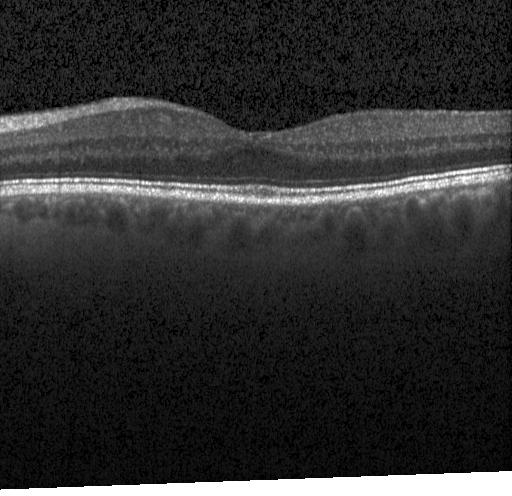

OCT line scan. Horizontal scan through the fovea. Heidelberg Spectralis. Dx: neither choroidal neovascularization, diabetic macular edema, nor drusen.